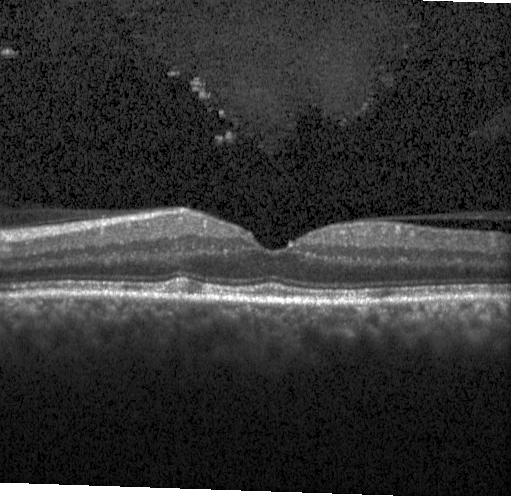 Impression: drusen.